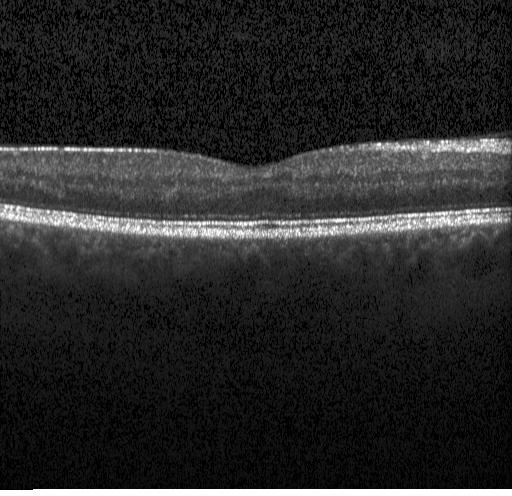

Spectral-domain optical coherence tomography; instrument: Heidelberg Spectralis; macular scan; retinal OCT B-scan
The scan shows no CNV, DME, or drusen.